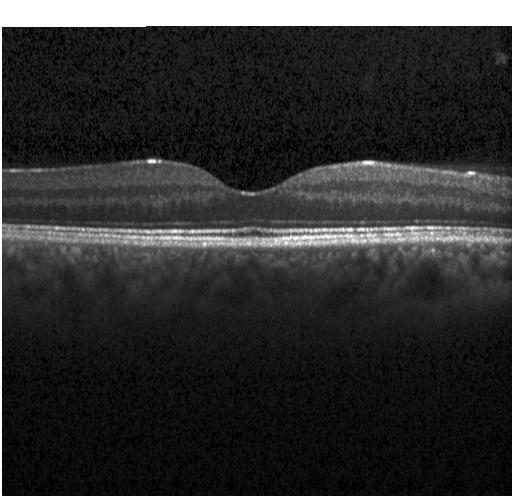 Impression: neither CNV, DME, nor drusen.